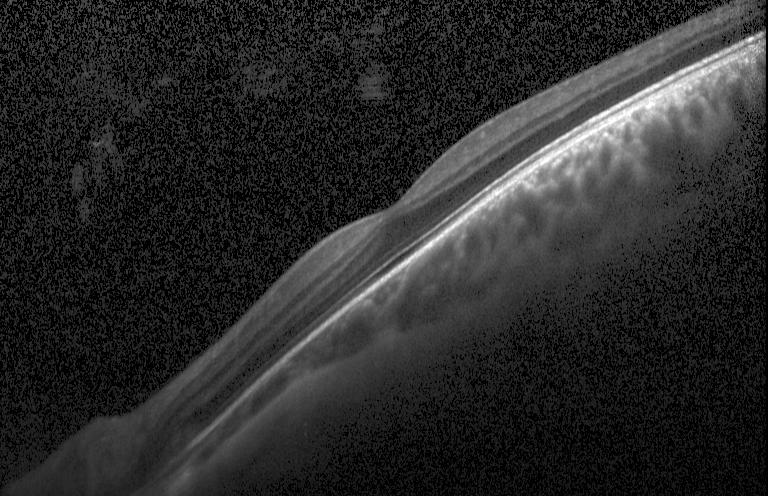 SD-OCT; instrument: Heidelberg Spectralis; OCT line scan — Assessment: neither choroidal neovascularization, diabetic macular edema, nor drusen.